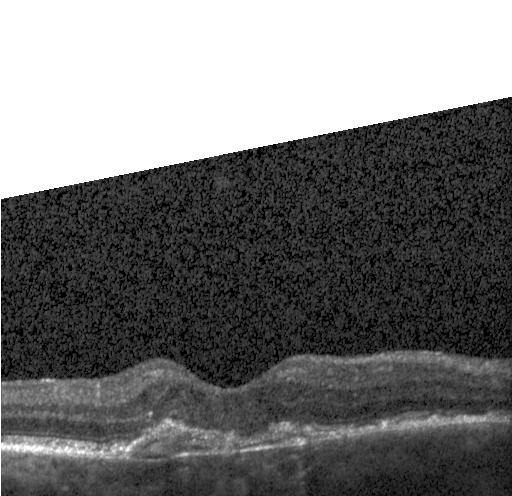
Retinal OCT B-scan, spectral-domain optical coherence tomography
Finding: a choroidal neovascular membrane.